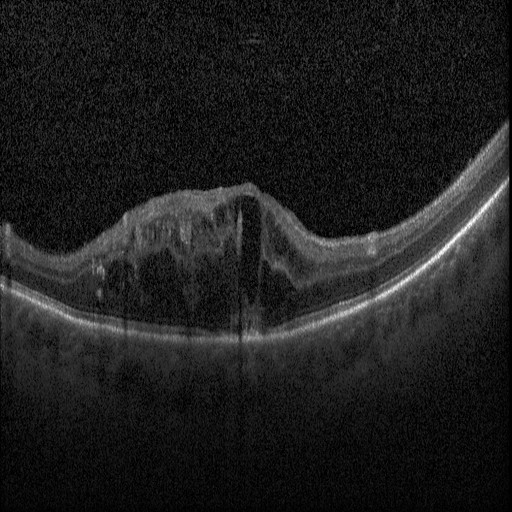 The scan shows DME.